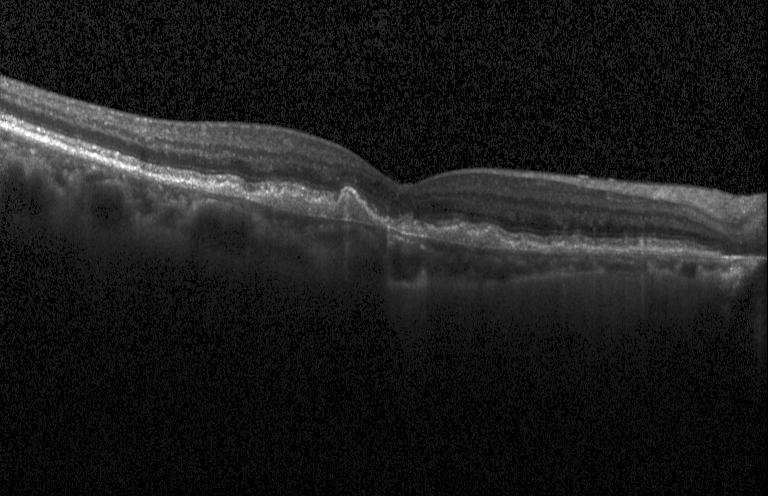

Macular OCT: choroidal neovascularization.